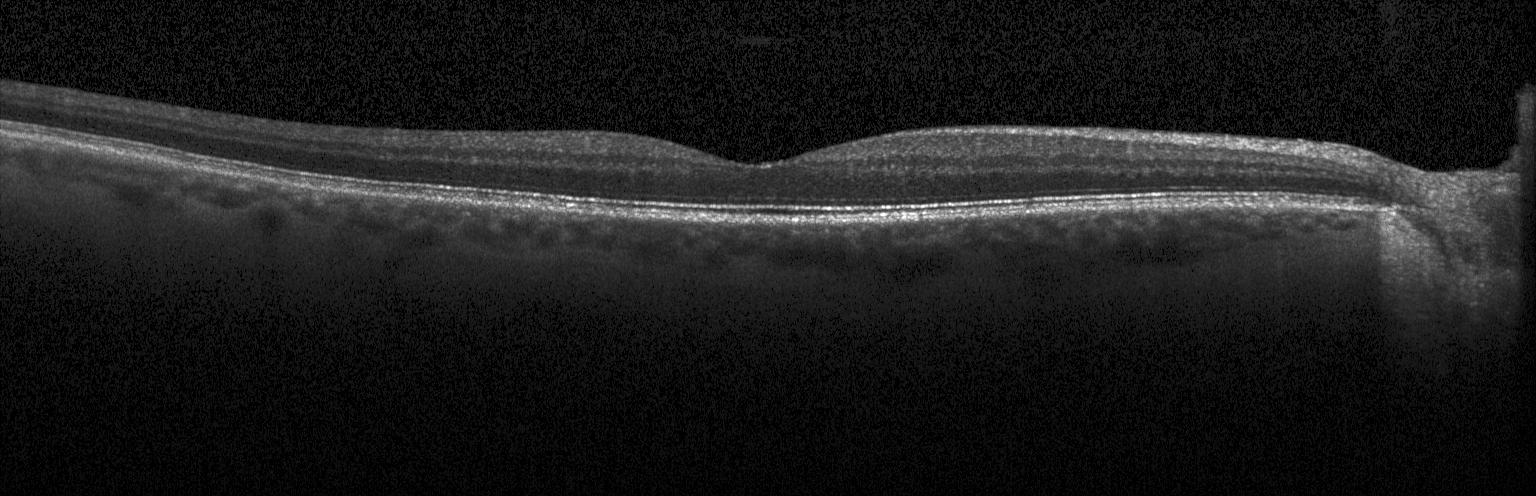 Acquired on a Heidelberg Spectralis · OCT line scan · spectral-domain optical coherence tomography.
Impression: no choroidal neovascularization, diabetic macular edema, or drusen.